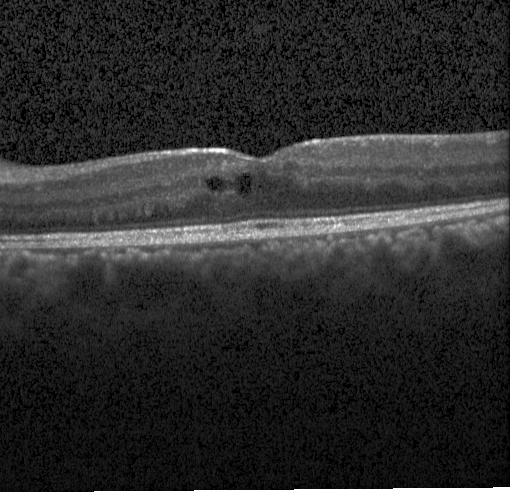 Retinal OCT B-scan; SD-OCT. Diagnosis: DME.